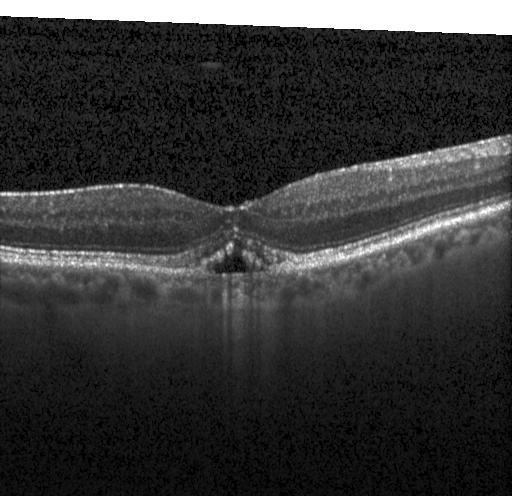
A choroidal neovascular membrane.